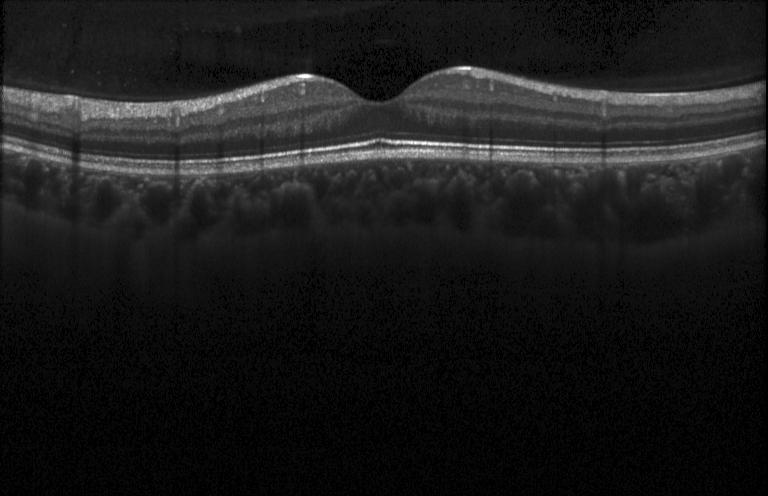 Optical coherence tomography scan. Assessment: no choroidal neovascularization, no diabetic macular edema, and no drusen.